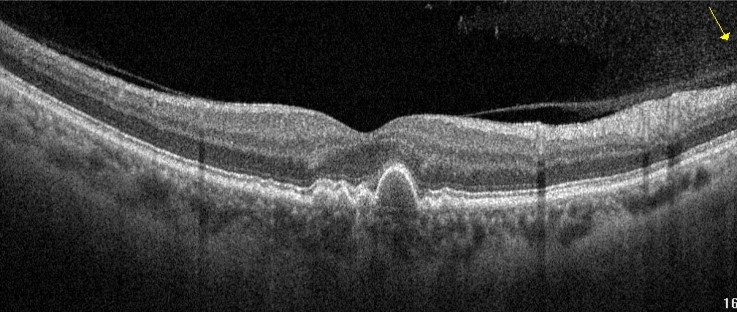

Optical coherence tomography B-scan · macular scan · acquired on an Optovue Avanti RTVue XR
Impression: age-related macular degeneration (AMD).